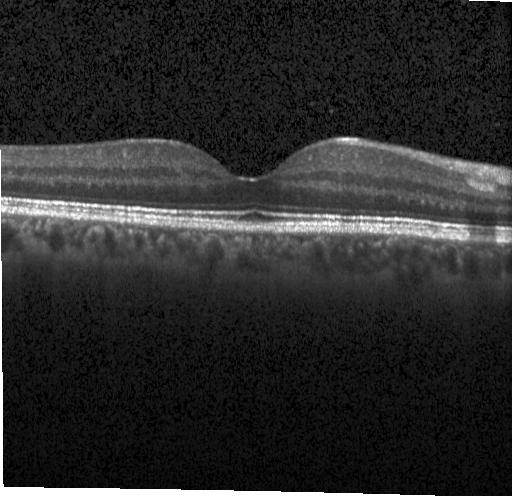

Finding: no choroidal neovascularization, diabetic macular edema, or drusen.